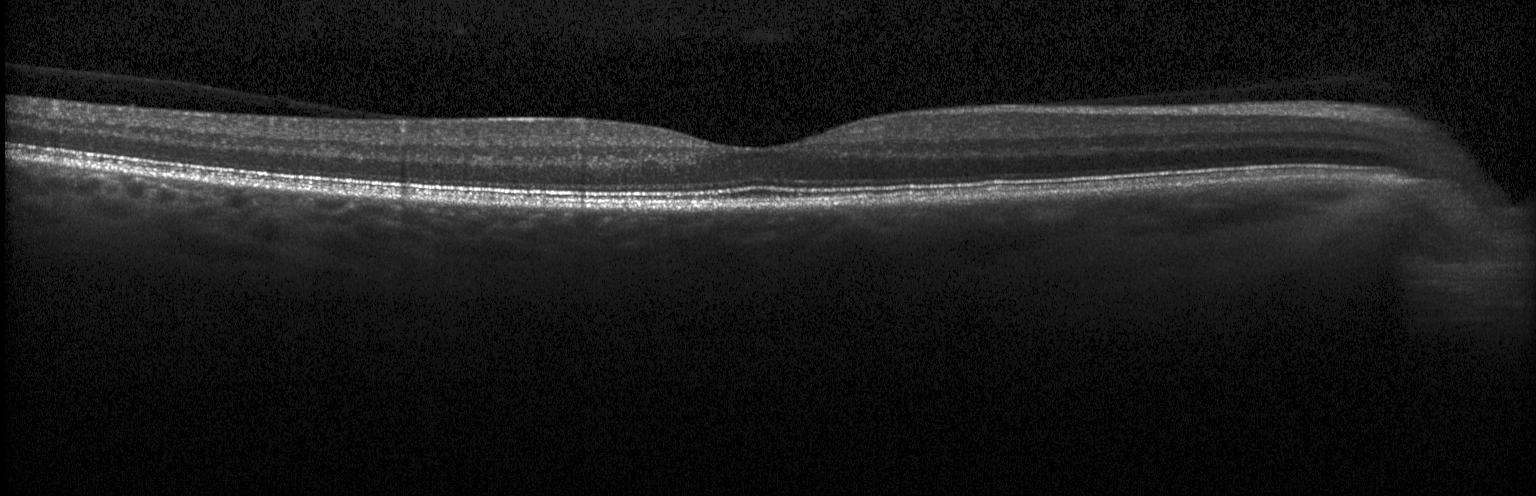
OCT finding: neither choroidal neovascularization, diabetic macular edema, nor drusen.